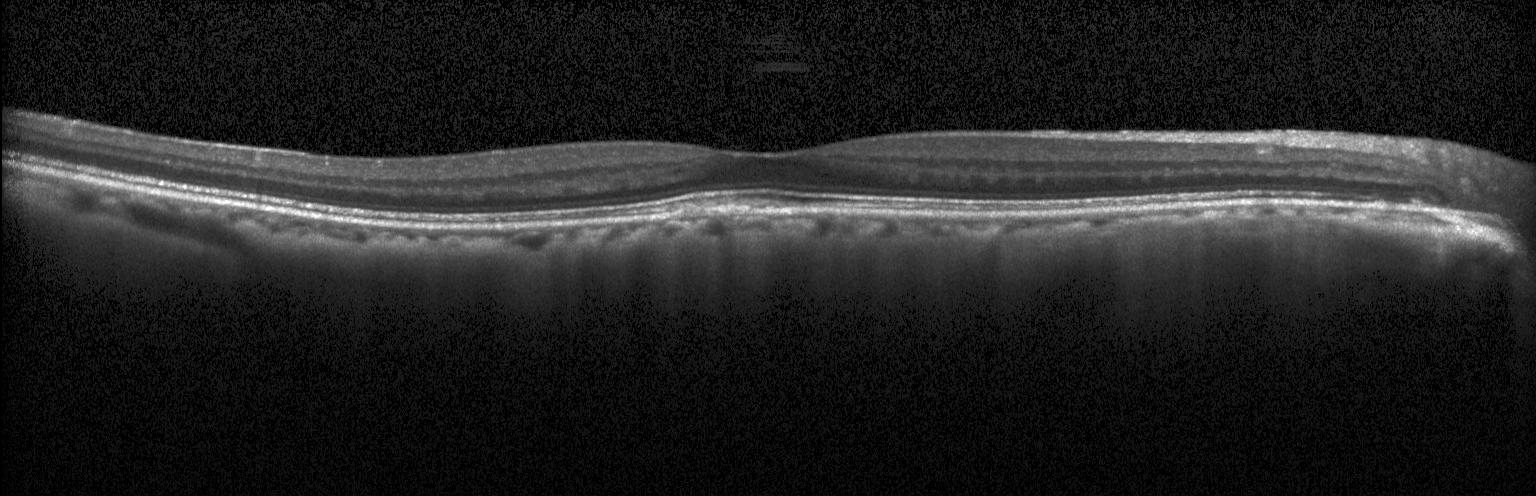 Spectral-domain optical coherence tomography, macular scan, retinal OCT B-scan. OCT finding: no CNV, DME, or drusen.